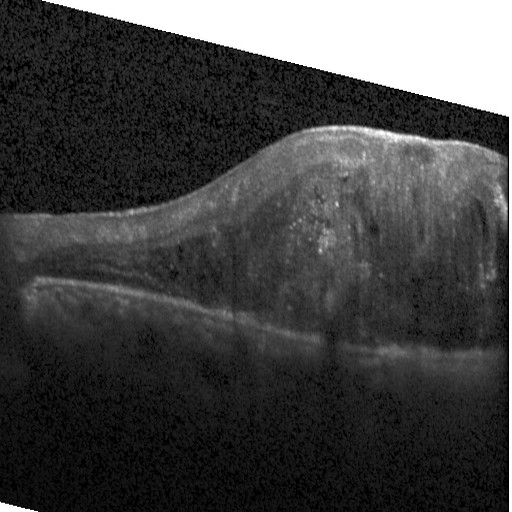

Heidelberg Spectralis OCT system. Retinal OCT cross-section.
Impression: DME.